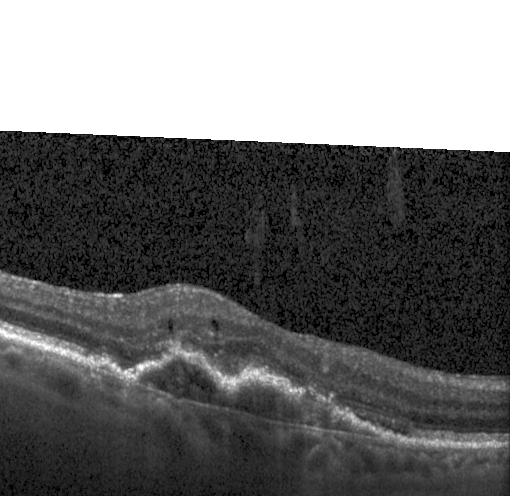 Spectral-domain optical coherence tomography · retinal OCT B-scan. Macular OCT: a choroidal neovascular membrane.